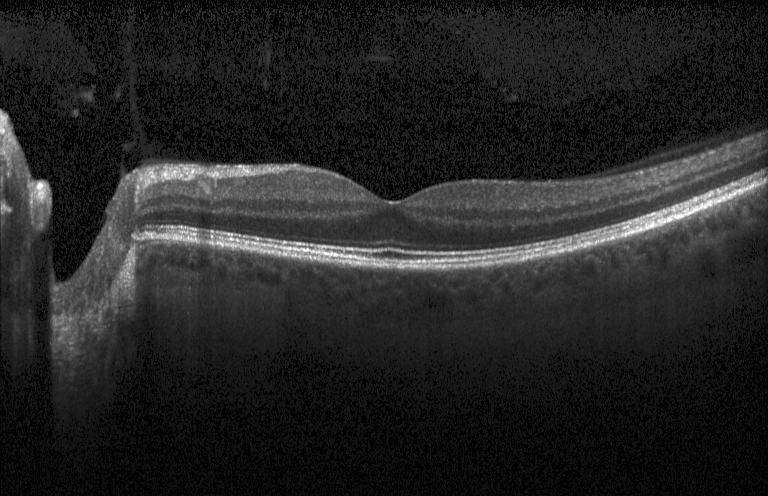 Acquired on a Heidelberg Spectralis; OCT B-scan; spectral-domain OCT.
No choroidal neovascularization, diabetic macular edema, or drusen.